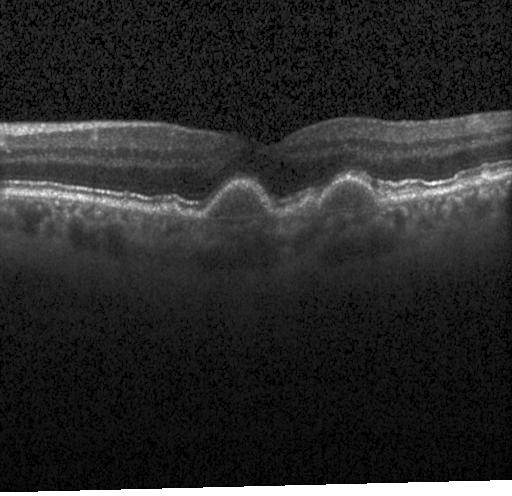
OCT finding: sub-RPE drusenoid deposits.